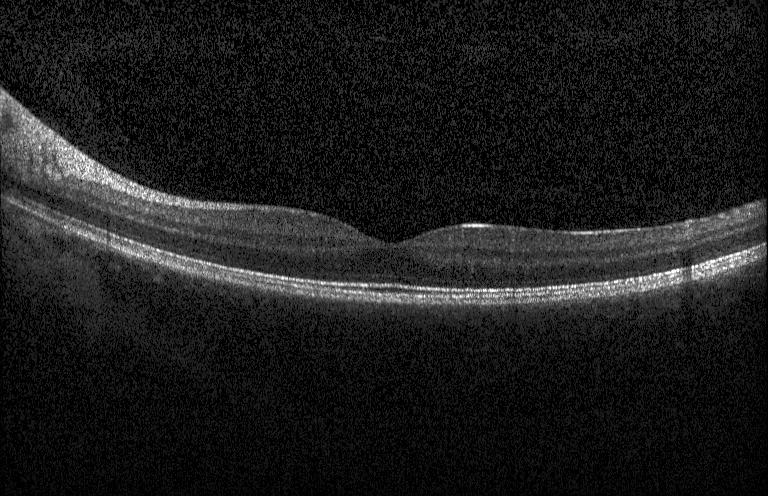
Retinal OCT B-scan; centered on the fovea — The scan shows no evidence of choroidal neovascularization, diabetic macular edema, or drusen.